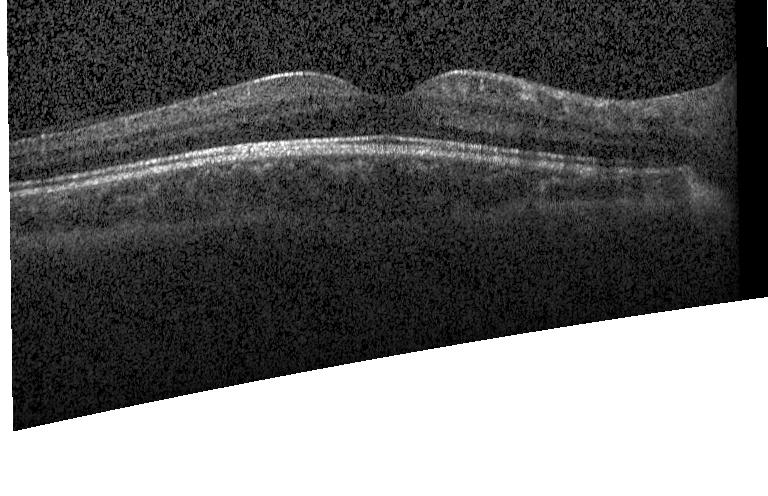

Macular scan, OCT B-scan, Heidelberg Spectralis OCT system
Finding: no choroidal neovascularization, no diabetic macular edema, and no drusen.